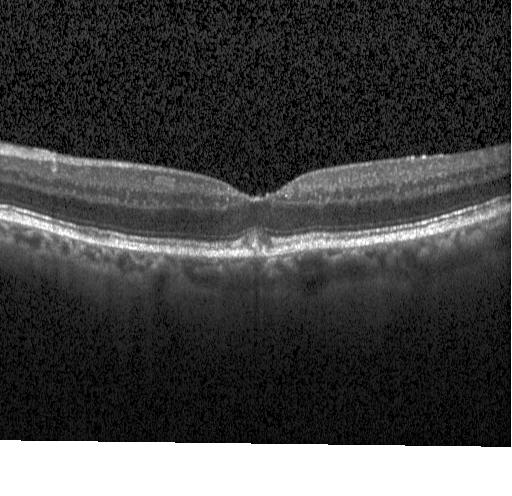 Retinal OCT cross-section showing sub-RPE drusenoid deposits.